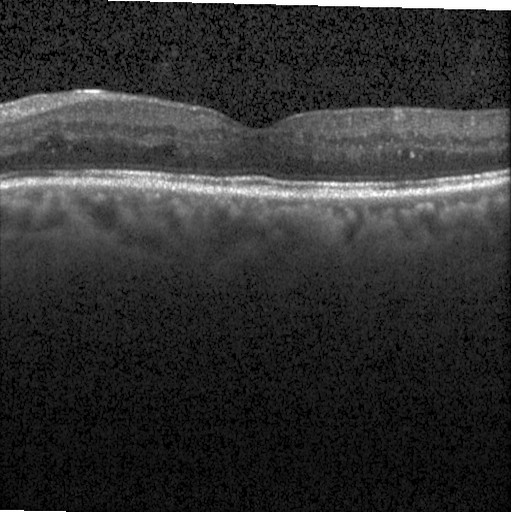
Optical coherence tomography scan — Impression: diabetic macular edema.